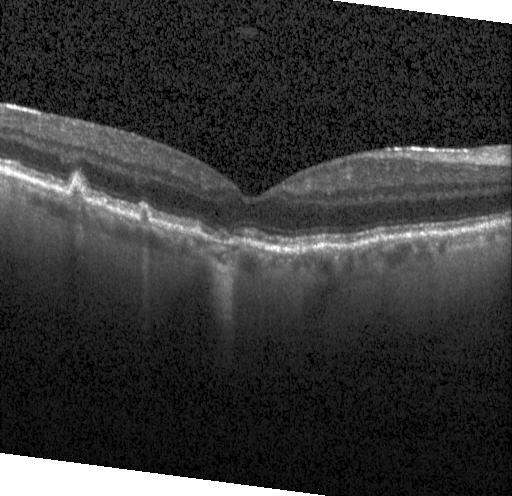
Finding: sub-RPE drusenoid deposits.